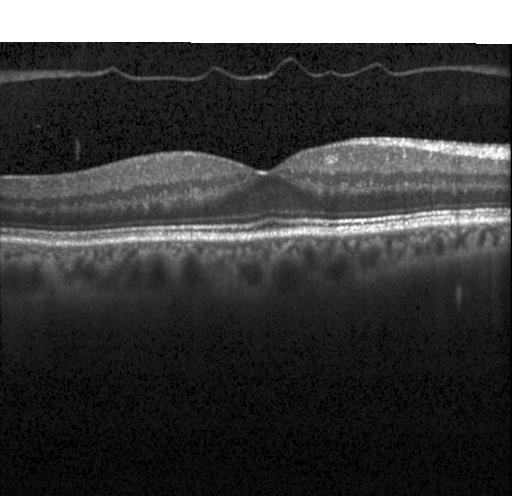

OCT B-scan. Through the macula. Spectral-domain OCT. Instrument: Heidelberg Spectralis — OCT finding: no choroidal neovascularization, no diabetic macular edema, and no drusen.